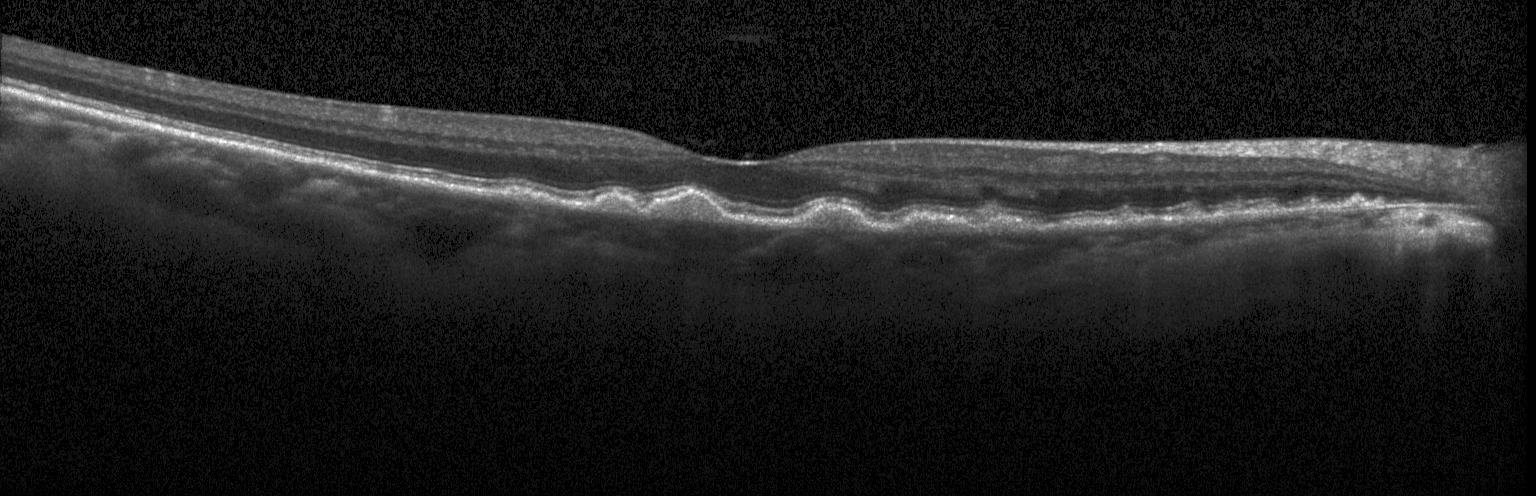
OCT B-scan, centered on the fovea — Finding: multiple drusen.